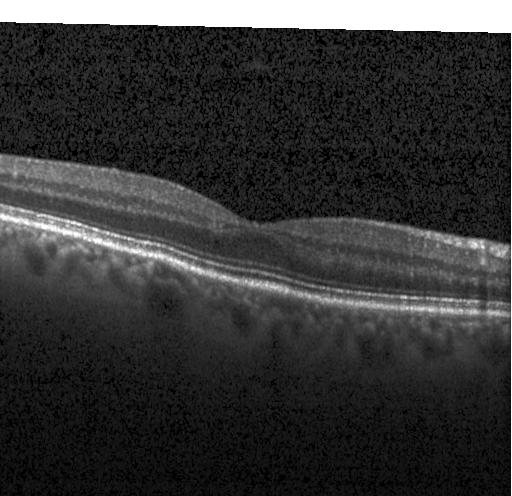
Acquired on a Heidelberg Spectralis · through the macula · OCT B-scan.
This B-scan demonstrates no choroidal neovascularization, diabetic macular edema, or drusen.